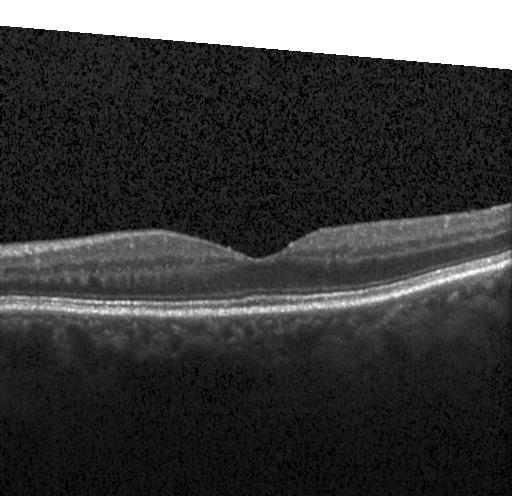 Spectral-domain optical coherence tomography; OCT B-scan; through the macula.
Assessment: neither choroidal neovascularization, diabetic macular edema, nor drusen.